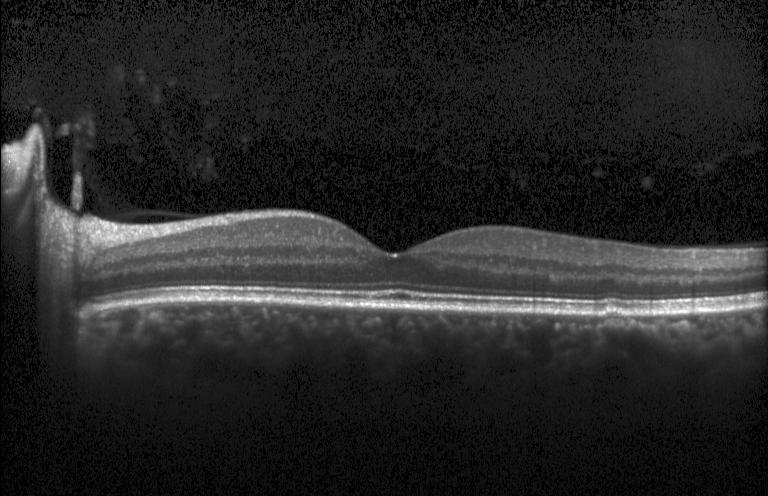 Instrument: Heidelberg Spectralis; fovea-centered; OCT B-scan; SD-OCT. Diagnosis: no choroidal neovascularization, diabetic macular edema, or drusen.